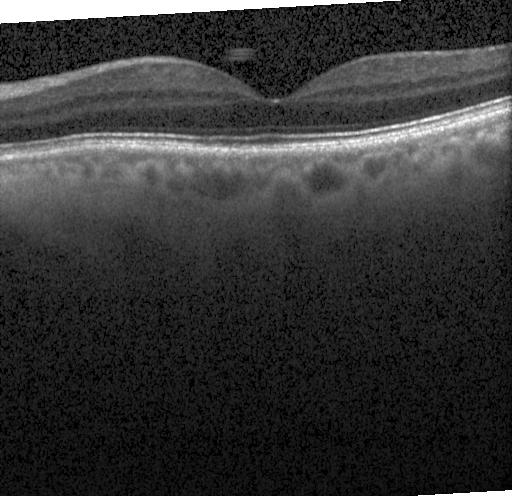
Through the macula · optical coherence tomography B-scan · acquired on a Heidelberg Spectralis.
This B-scan demonstrates no CNV, no DME, and no drusen.